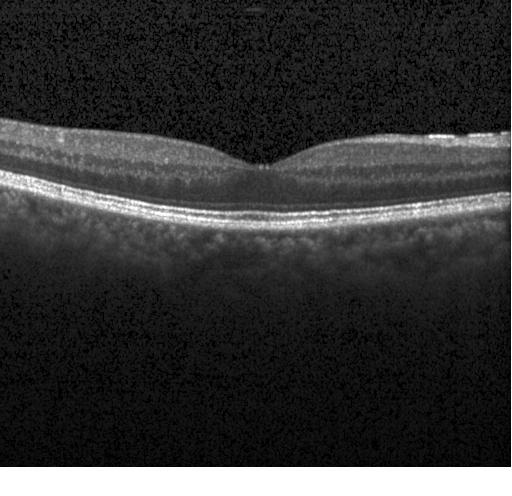
Heidelberg Spectralis OCT system. Retinal OCT cross-section. Centered on the fovea. Assessment: no CNV, DME, or drusen.